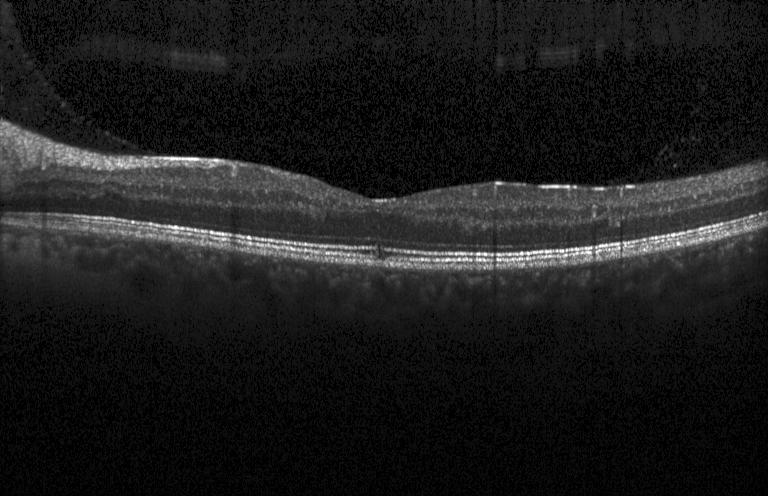
SD-OCT · instrument: Heidelberg Spectralis · OCT B-scan. Diagnosis: neither choroidal neovascularization, diabetic macular edema, nor drusen.